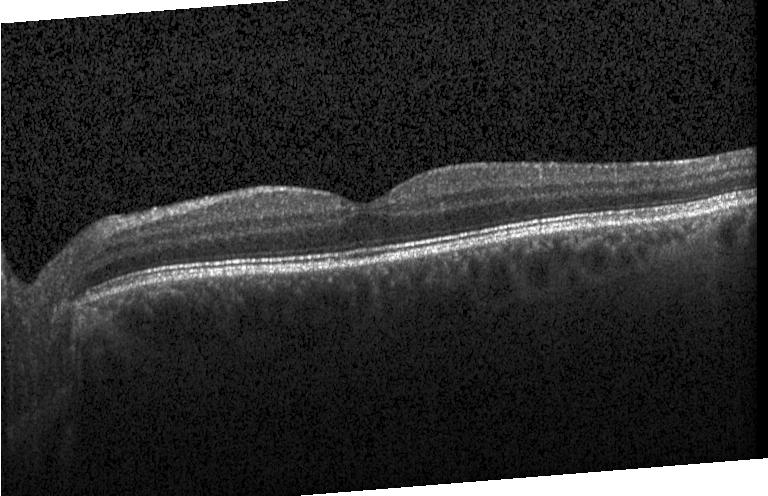

Finding: no choroidal neovascularization, diabetic macular edema, or drusen.